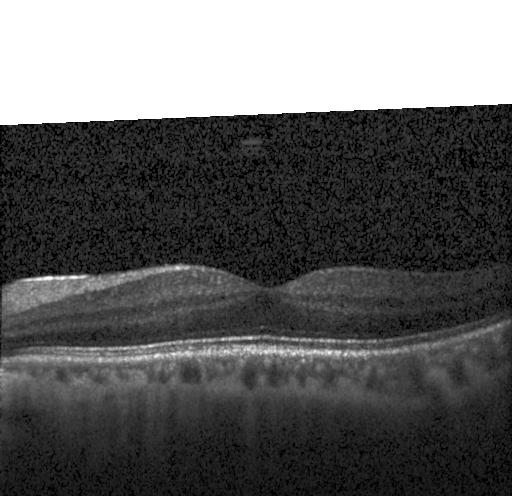 OCT line scan. SD-OCT. Heidelberg Spectralis. Impression: no CNV, DME, or drusen.